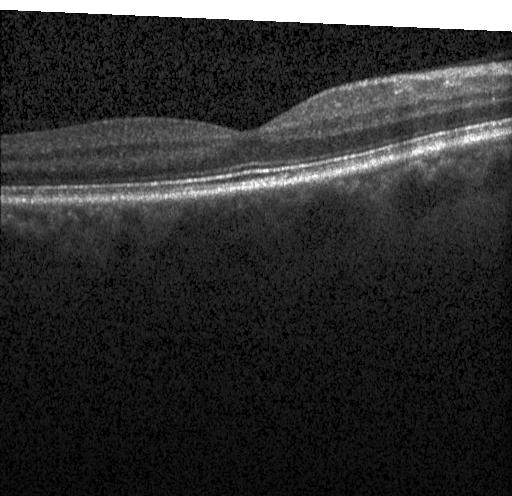
Optical coherence tomography B-scan — Finding: no evidence of choroidal neovascularization, diabetic macular edema, or drusen.